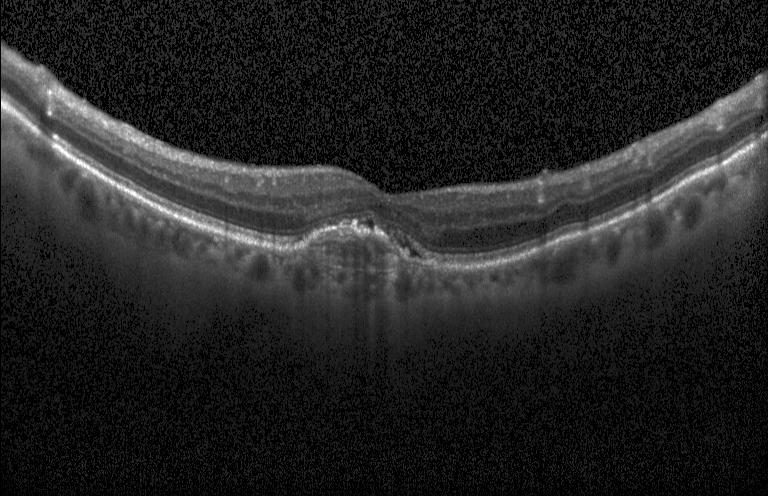 Spectral-domain OCT. Optical coherence tomography scan. Macular scan. Acquired on a Heidelberg Spectralis — Impression: a choroidal neovascular membrane.